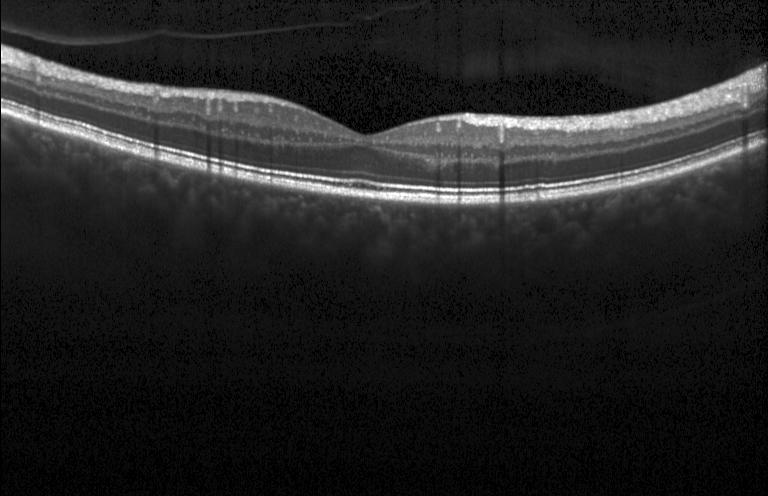
Macular scan; SD-OCT; OCT B-scan; Heidelberg Spectralis — Assessment: no evidence of choroidal neovascularization, diabetic macular edema, or drusen.